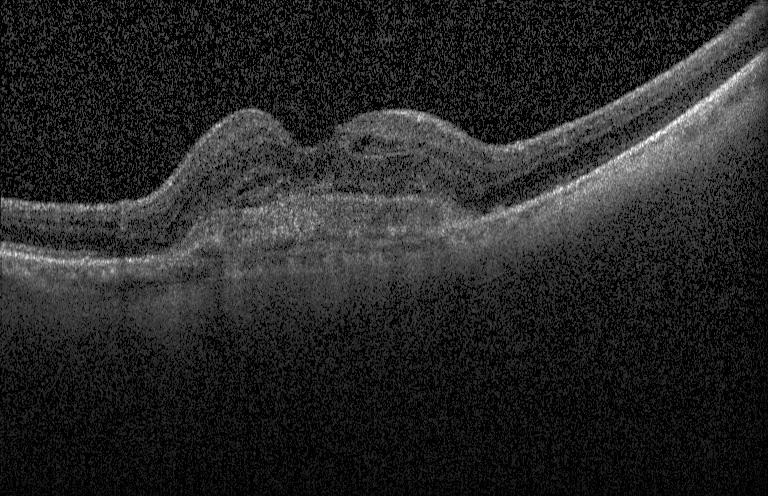

Macular scan · retinal OCT cross-section · Heidelberg Spectralis OCT system · spectral-domain OCT.
Assessment: a choroidal neovascular membrane.